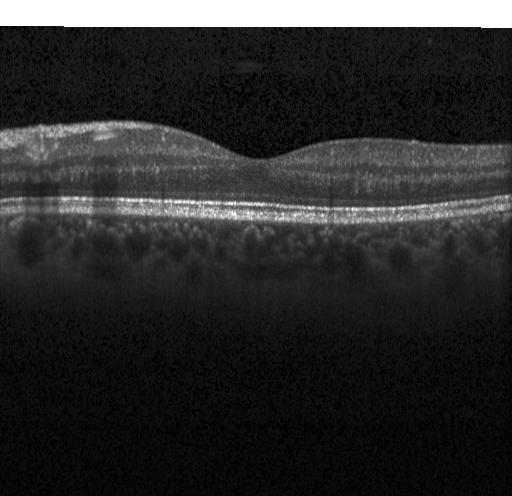
Retinal OCT B-scan
Assessment: no evidence of CNV, DME, or drusen.